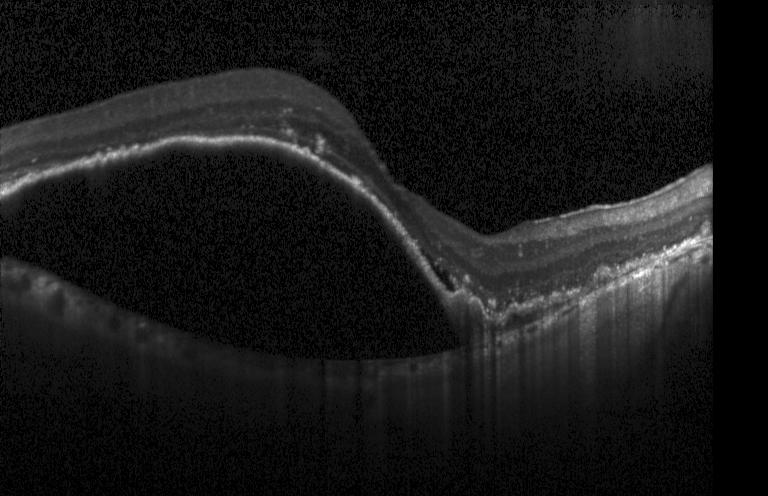
Impression: a choroidal neovascular membrane.